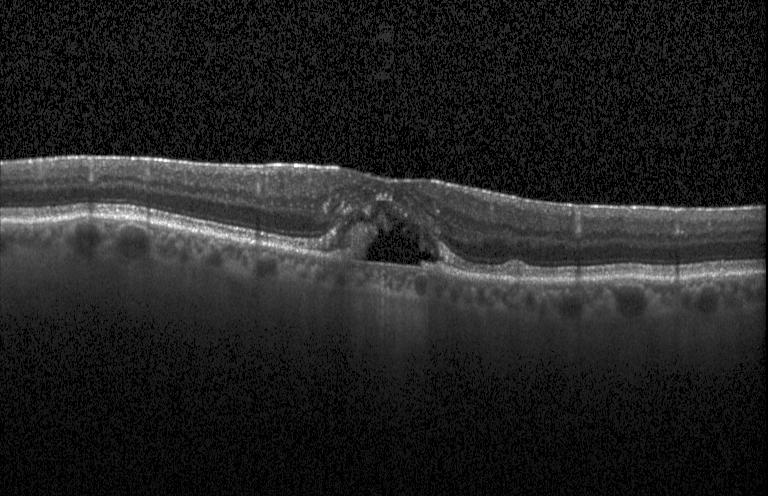
OCT line scan; acquired on a Heidelberg Spectralis — OCT finding: a choroidal neovascular membrane.